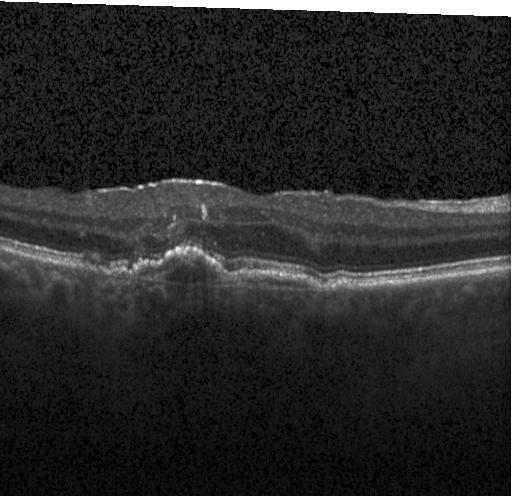

Optical coherence tomography B-scan.
Finding: a choroidal neovascular membrane.